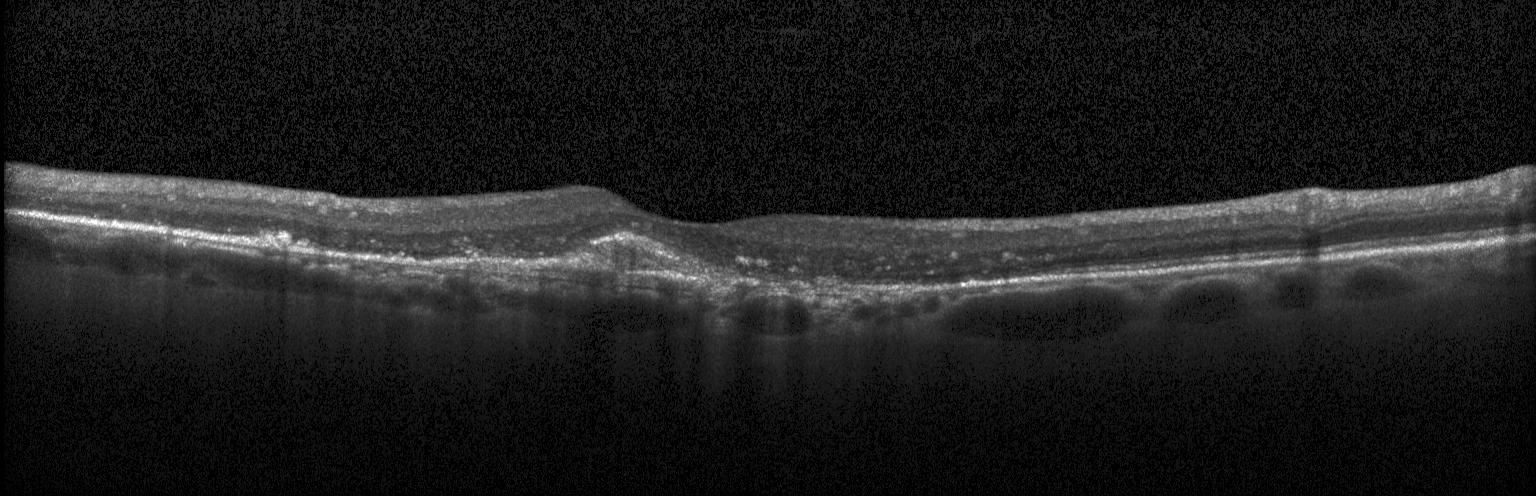

Fovea-centered, retinal OCT B-scan
Finding: choroidal neovascularization (CNV).